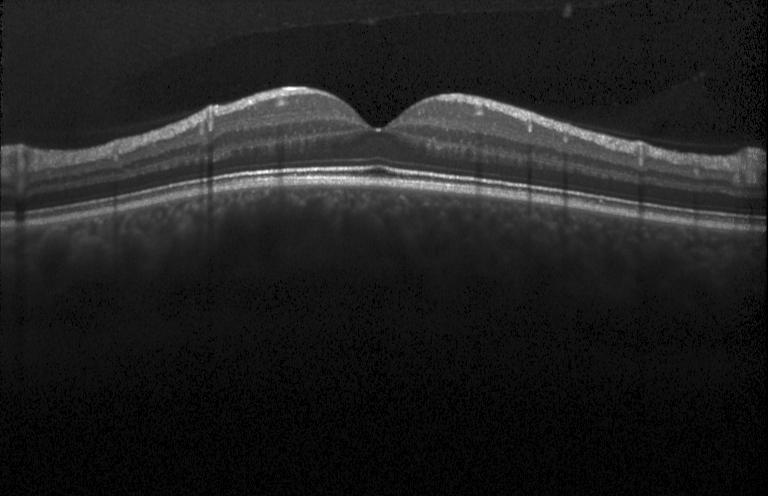
No evidence of CNV, DME, or drusen.